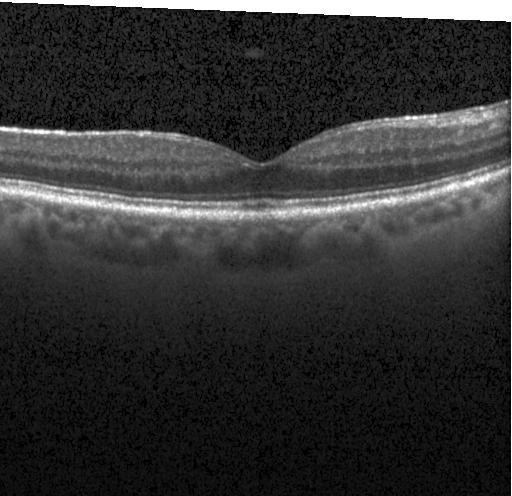

Impression: no evidence of choroidal neovascularization, diabetic macular edema, or drusen.